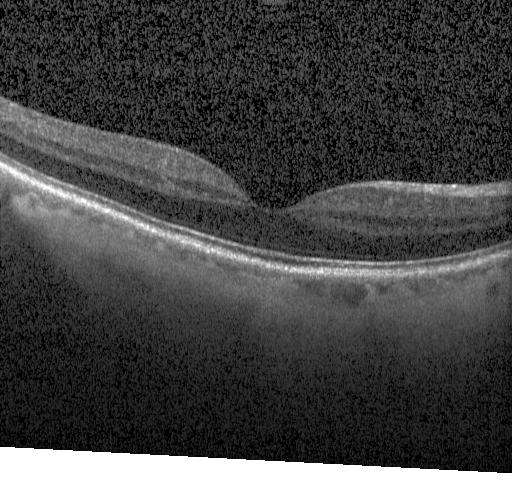 OCT B-scan; macular scan; spectral-domain optical coherence tomography.
Finding: neither choroidal neovascularization, diabetic macular edema, nor drusen.